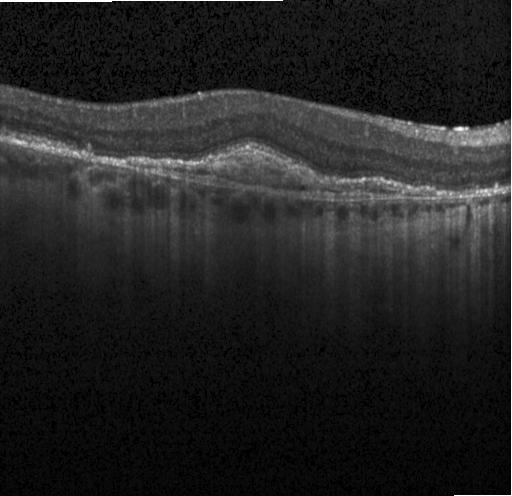 OCT B-scan; Heidelberg Spectralis; horizontal scan through the fovea
This B-scan demonstrates a choroidal neovascular membrane.